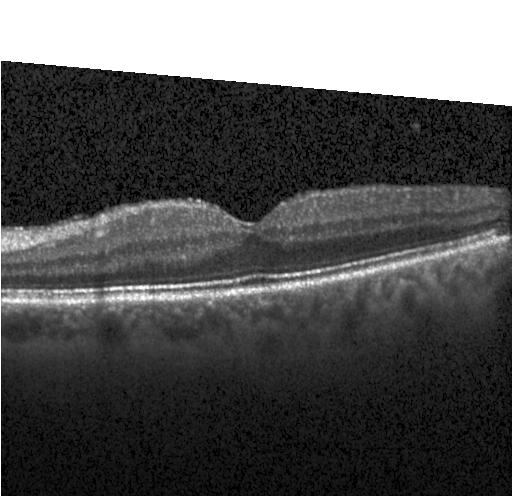

Assessment: no CNV, no DME, and no drusen.